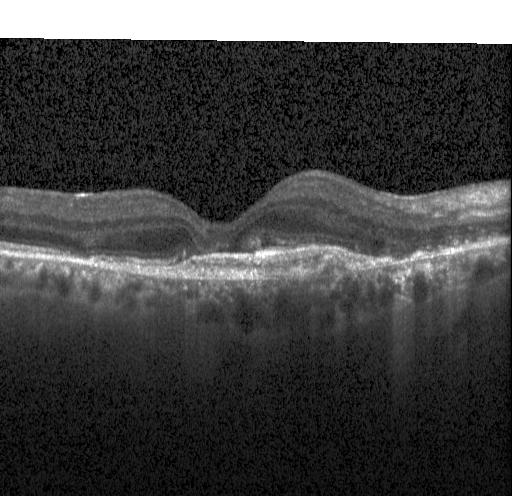
Retinal OCT cross-section · SD-OCT · Heidelberg Spectralis — The scan shows choroidal neovascularization (CNV).